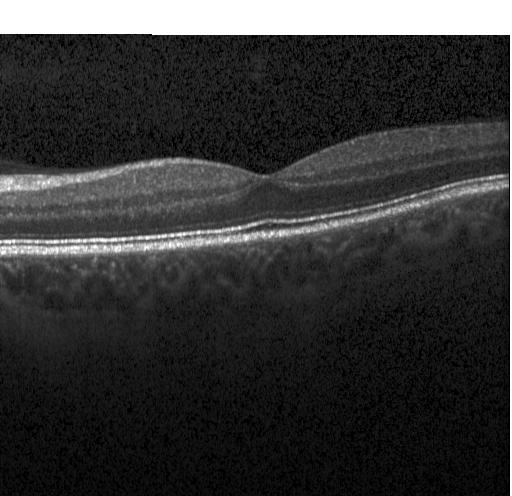
Spectral-domain optical coherence tomography. Optical coherence tomography scan. Instrument: Heidelberg Spectralis
Diagnosis: no CNV, DME, or drusen.